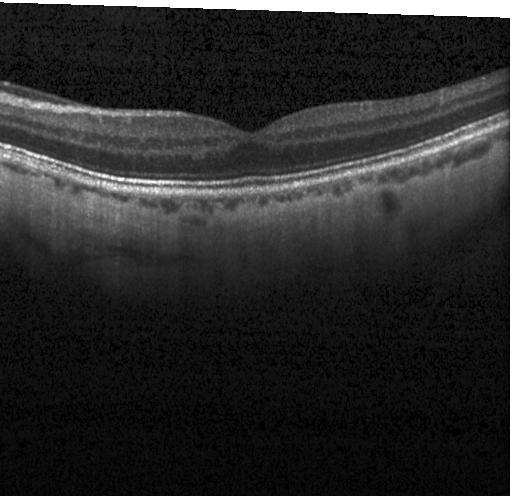
OCT scan showing no choroidal neovascularization, no diabetic macular edema, and no drusen.